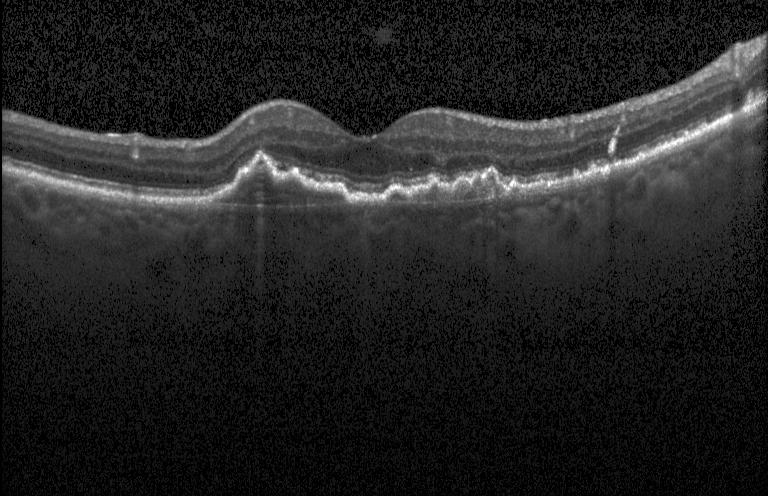
Acquired on a Heidelberg Spectralis; OCT line scan. CNV.